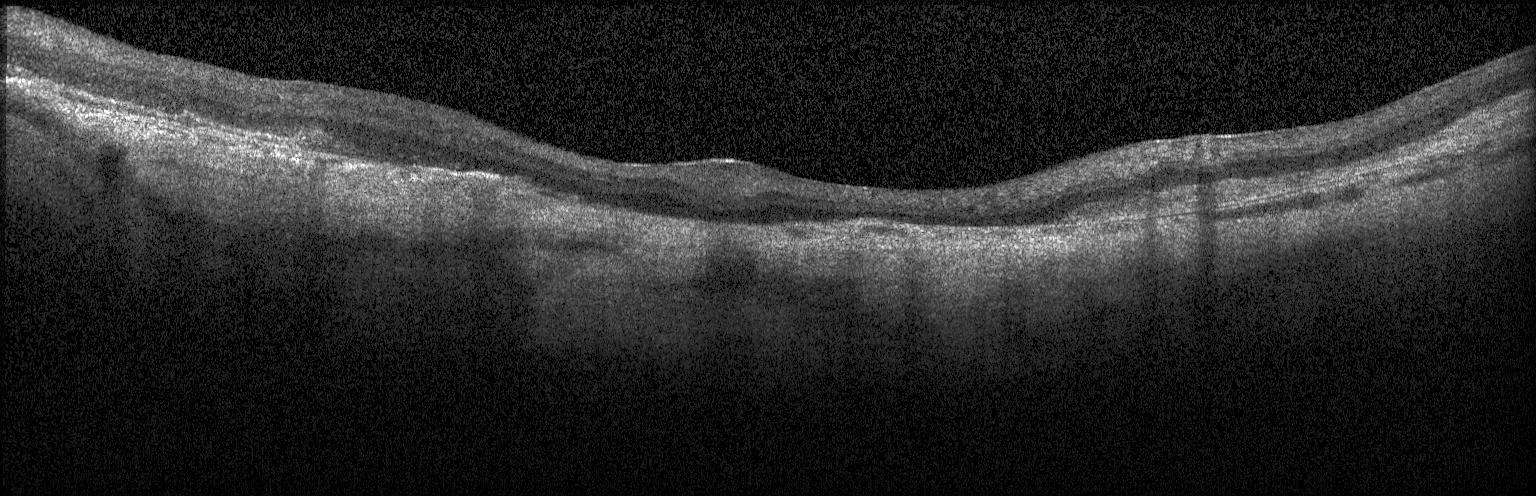
Retinal OCT B-scan
This B-scan demonstrates a choroidal neovascular membrane.